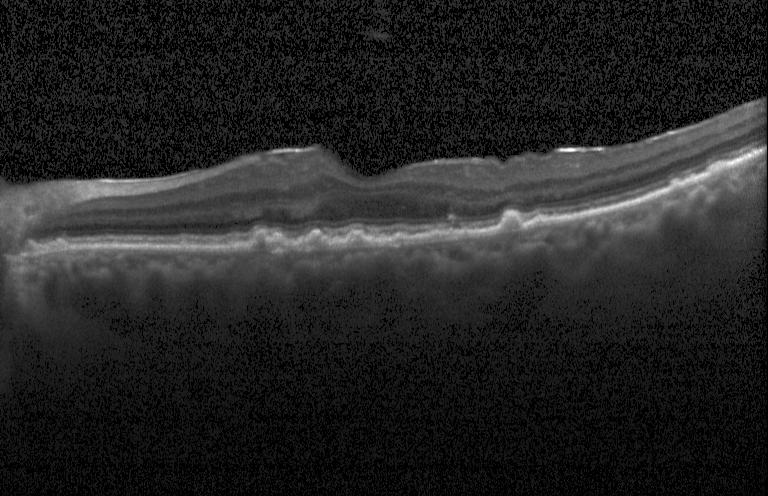 Horizontal scan through the fovea. Heidelberg Spectralis OCT system. SD-OCT. Retinal OCT cross-section. The scan shows drusen.